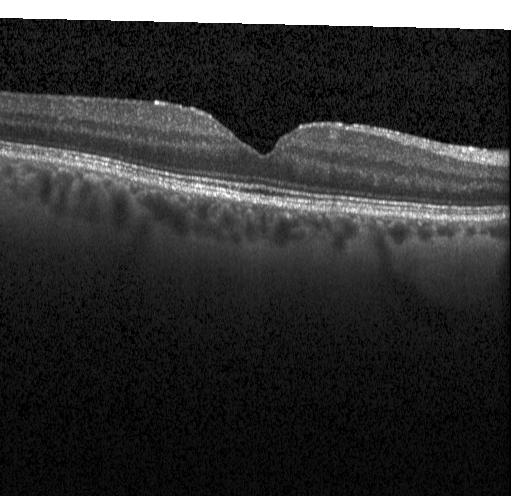 Retinal OCT cross-section, Heidelberg Spectralis OCT system, horizontal scan through the fovea, SD-OCT.
Impression: neither choroidal neovascularization, diabetic macular edema, nor drusen.